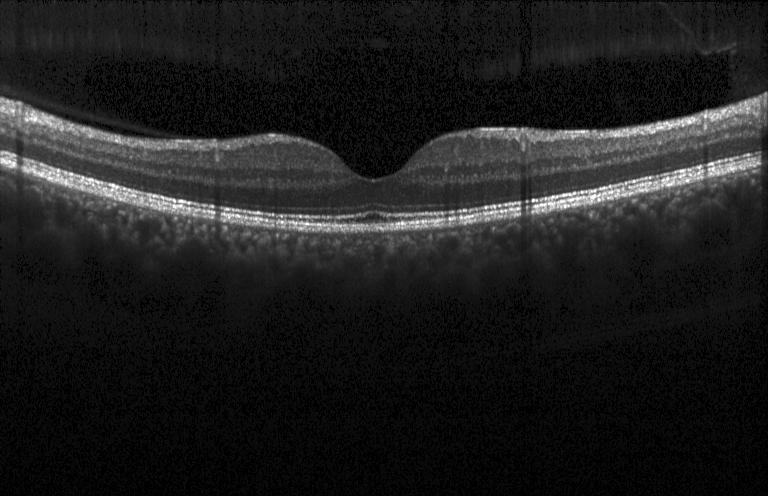
Diagnosis: no CNV, no DME, and no drusen.